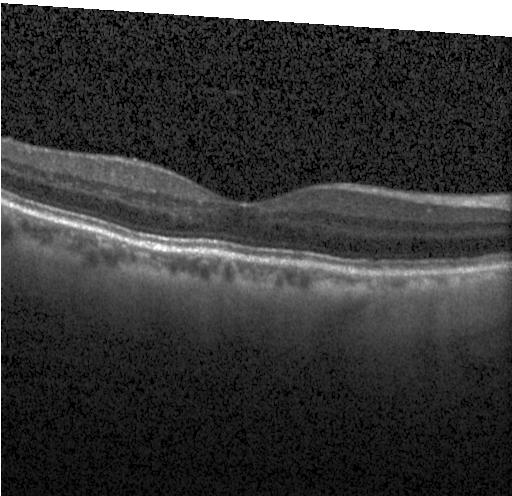
OCT B-scan · horizontal scan through the fovea
Impression: neither CNV, DME, nor drusen.